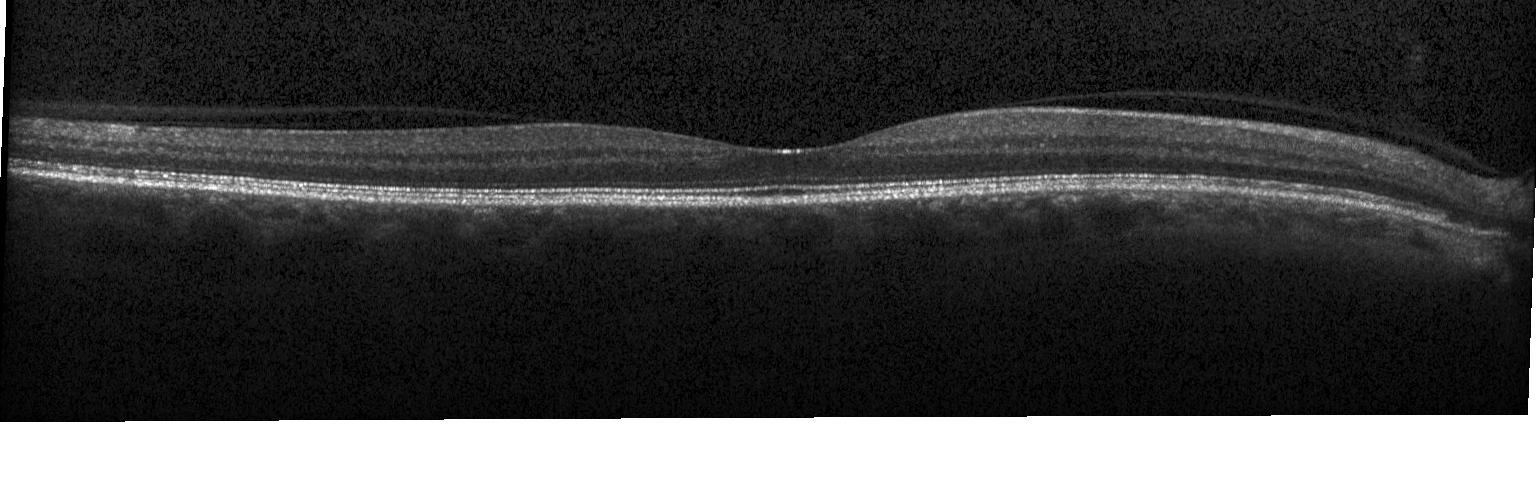

OCT B-scan showing neither choroidal neovascularization, diabetic macular edema, nor drusen.